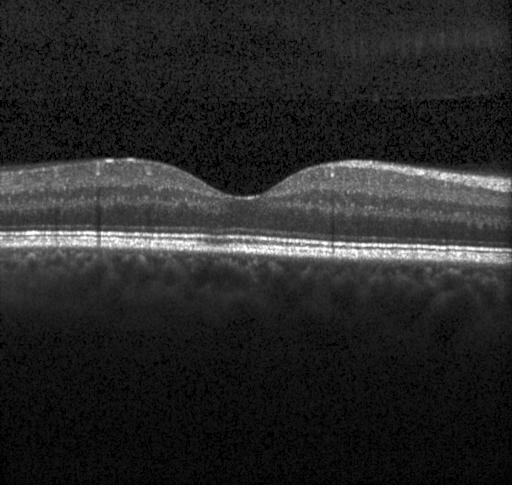
OCT scan showing no CNV, DME, or drusen.